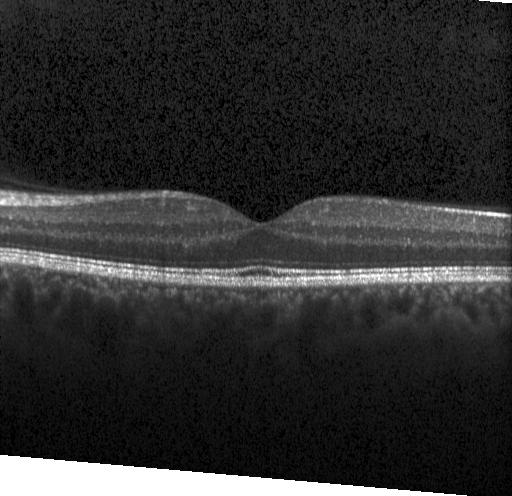

OCT B-scan, Heidelberg Spectralis OCT system, fovea-centered.
Macular OCT: no CNV, no DME, and no drusen.